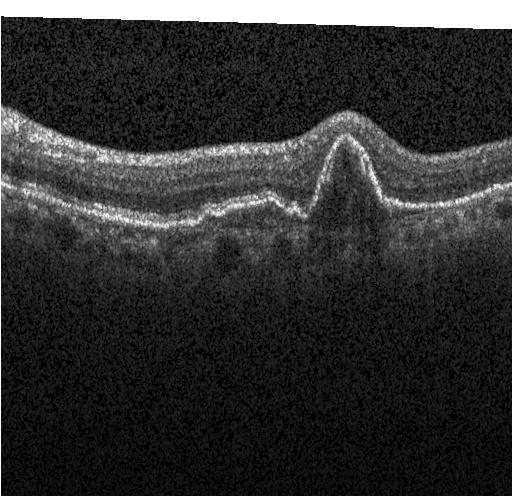
Spectral-domain OCT B-scan: a choroidal neovascular membrane.